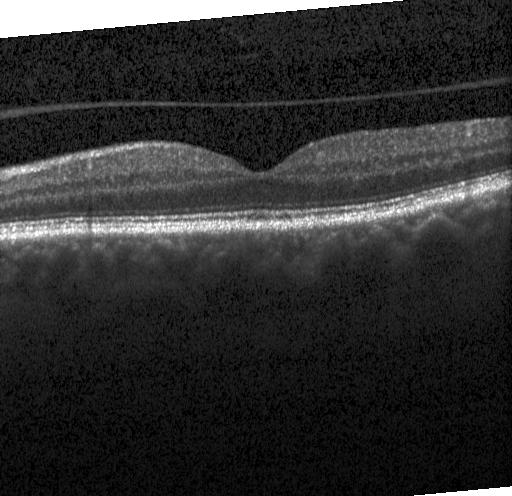 Spectral-domain optical coherence tomography · optical coherence tomography scan — Dx: no evidence of choroidal neovascularization, diabetic macular edema, or drusen.